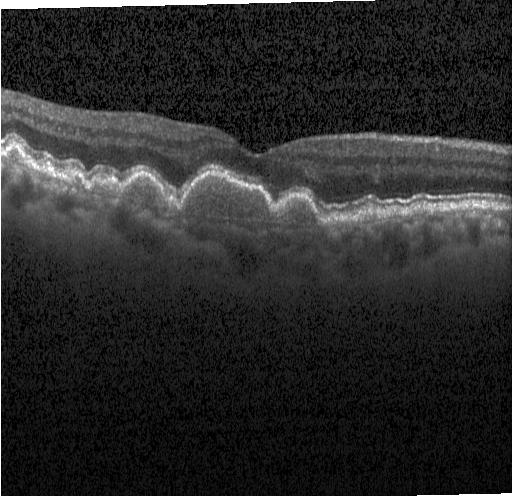

Retinal OCT B-scan; spectral-domain OCT; Heidelberg Spectralis; centered on the fovea.
Diagnosis: drusen.